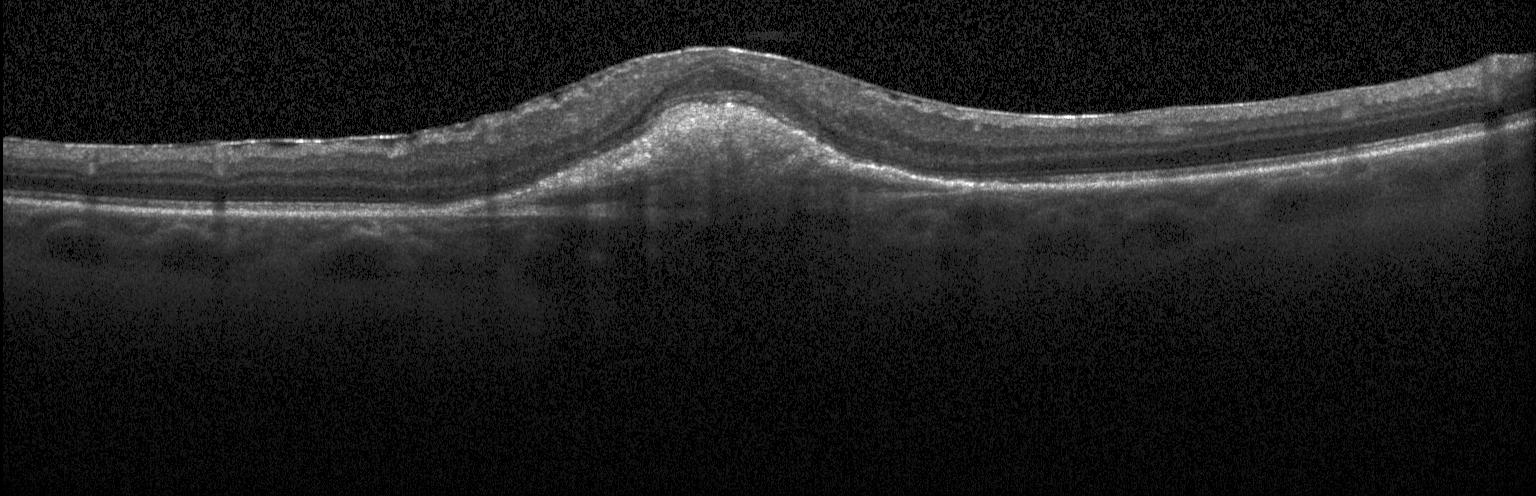 Spectral-domain optical coherence tomography. Acquired on a Heidelberg Spectralis. Optical coherence tomography B-scan. Through the macula
Dx: a choroidal neovascular membrane.